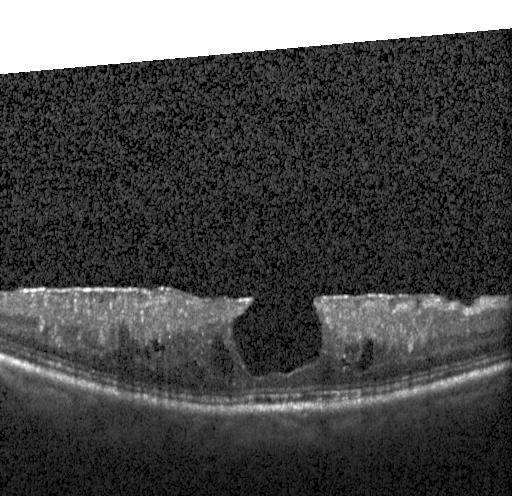 OCT line scan · through the macula · spectral-domain OCT · acquired on a Heidelberg Spectralis — Macular OCT: DME.